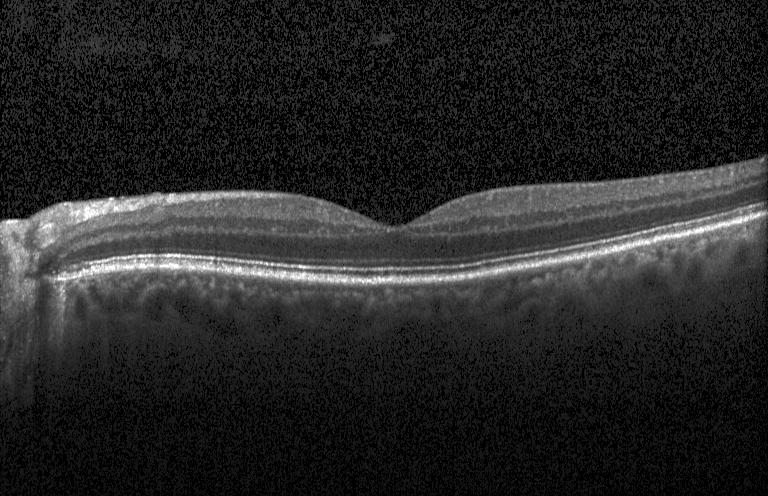 Dx: no choroidal neovascularization, diabetic macular edema, or drusen.